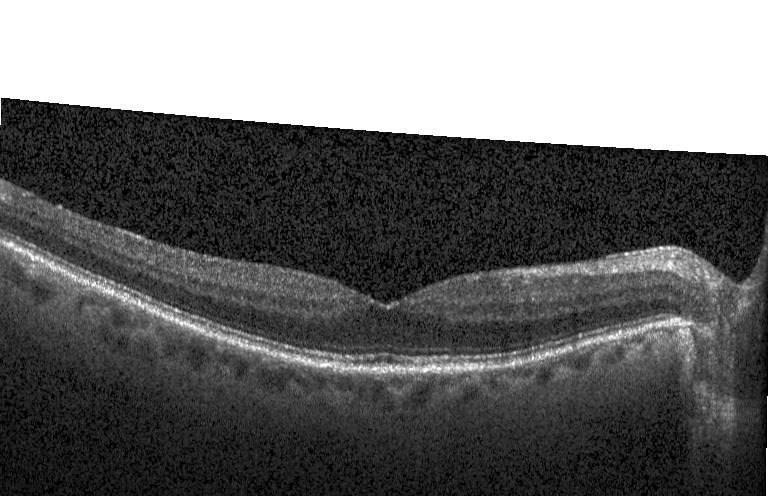

Optical coherence tomography B-scan.
Neither CNV, DME, nor drusen.